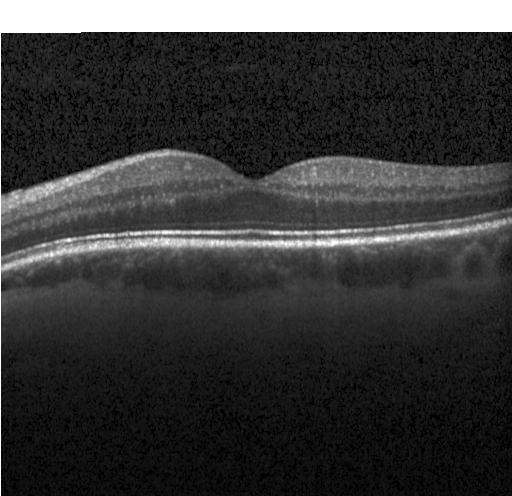 Spectral-domain optical coherence tomography, instrument: Heidelberg Spectralis, macular scan, OCT line scan. Assessment: neither choroidal neovascularization, diabetic macular edema, nor drusen.